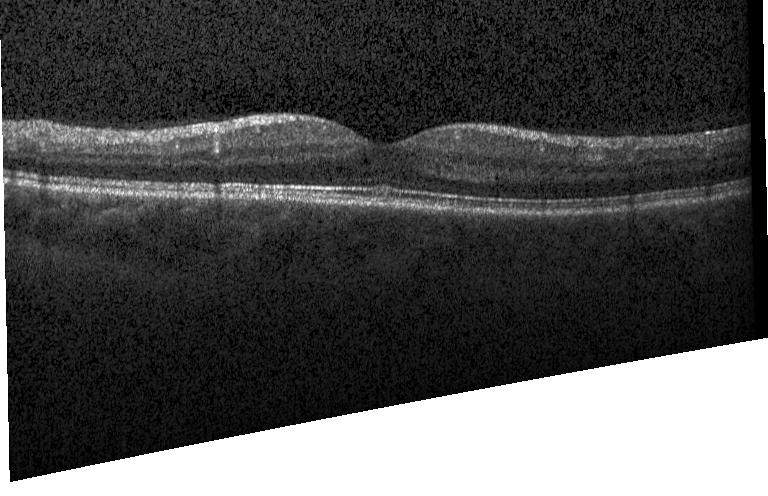 Instrument: Heidelberg Spectralis, macular scan, spectral-domain OCT, optical coherence tomography scan
This B-scan demonstrates no evidence of choroidal neovascularization, diabetic macular edema, or drusen.